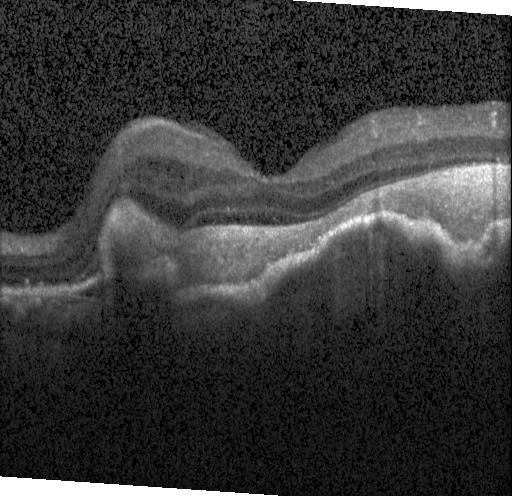 Diagnosis: a choroidal neovascular membrane.